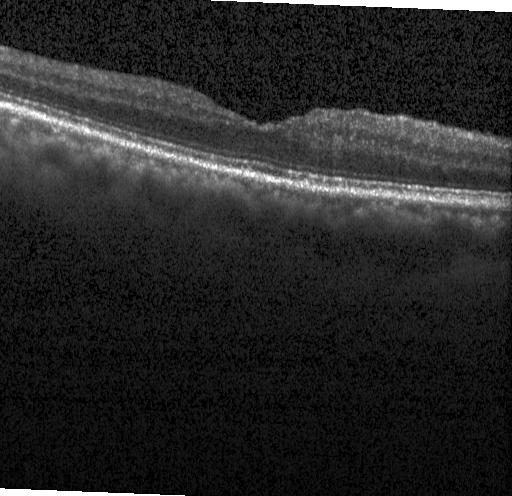 Dx: no choroidal neovascularization, no diabetic macular edema, and no drusen.